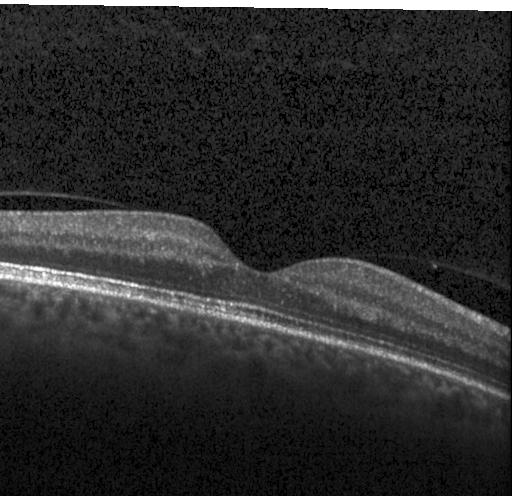 Acquired on a Heidelberg Spectralis, SD-OCT, optical coherence tomography B-scan.
The scan shows neither choroidal neovascularization, diabetic macular edema, nor drusen.